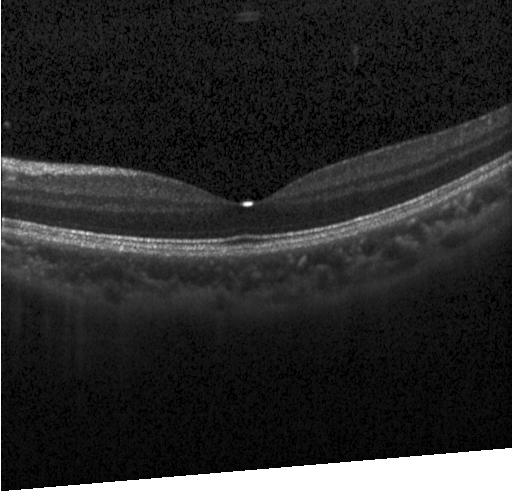 Heidelberg Spectralis. OCT B-scan. Spectral-domain OCT. Diagnosis: no choroidal neovascularization, diabetic macular edema, or drusen.